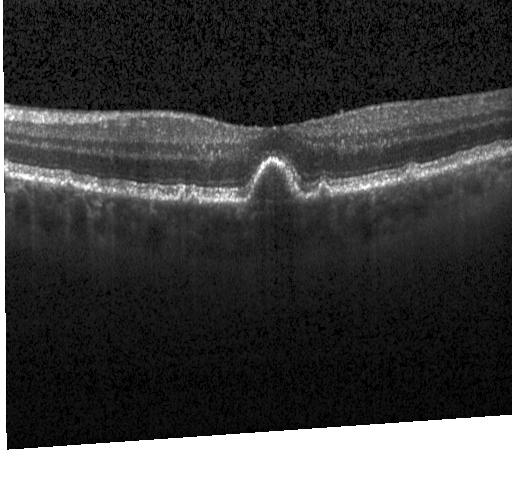 Spectral-domain optical coherence tomography; OCT B-scan. Impression: sub-RPE drusenoid deposits.